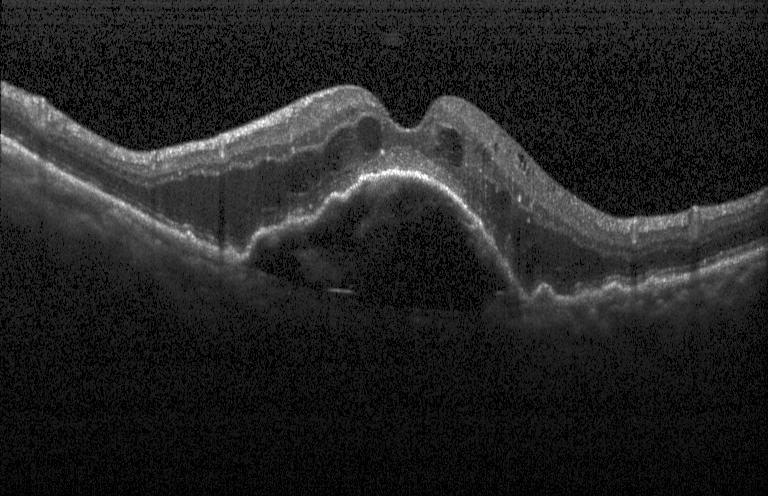
Instrument: Heidelberg Spectralis. Retinal OCT B-scan. Spectral-domain OCT. Fovea-centered. Finding: a choroidal neovascular membrane.